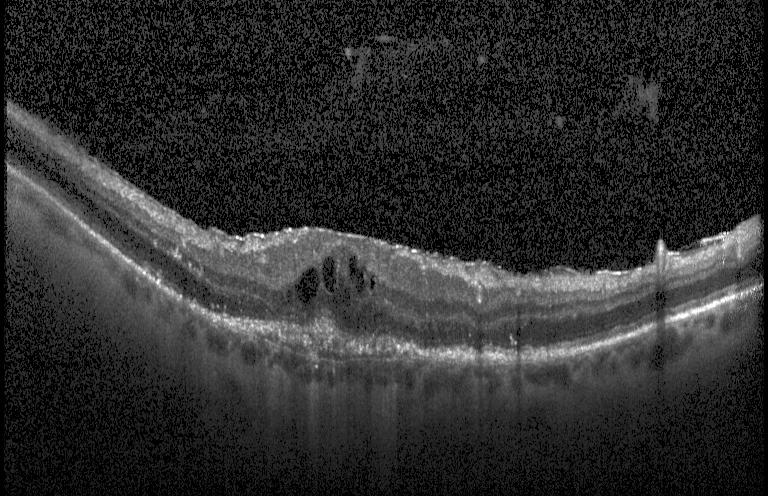

Heidelberg Spectralis OCT system; spectral-domain optical coherence tomography; optical coherence tomography B-scan. The scan shows a choroidal neovascular membrane.